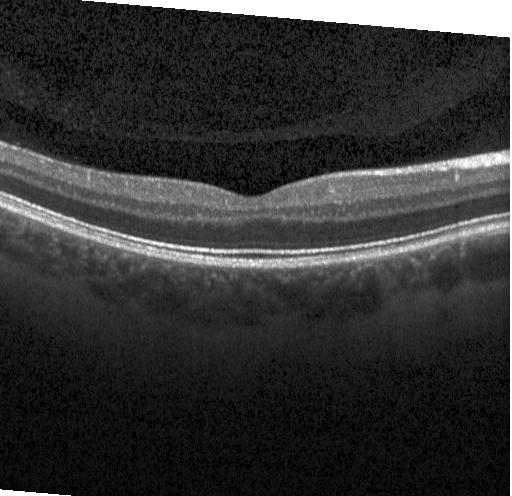

Spectral-domain OCT, instrument: Heidelberg Spectralis, macular scan, optical coherence tomography scan
Finding: no CNV, no DME, and no drusen.